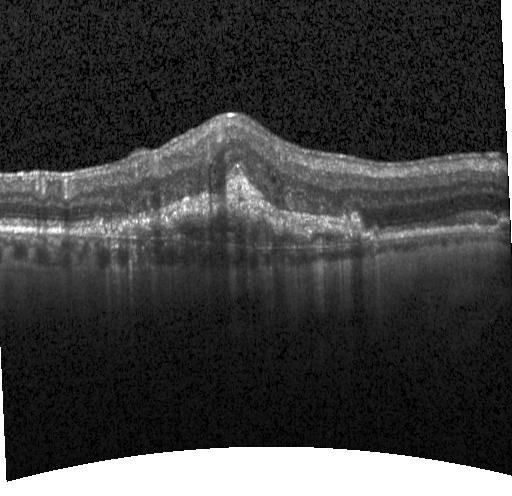
Optical coherence tomography B-scan.
Finding: a choroidal neovascular membrane.